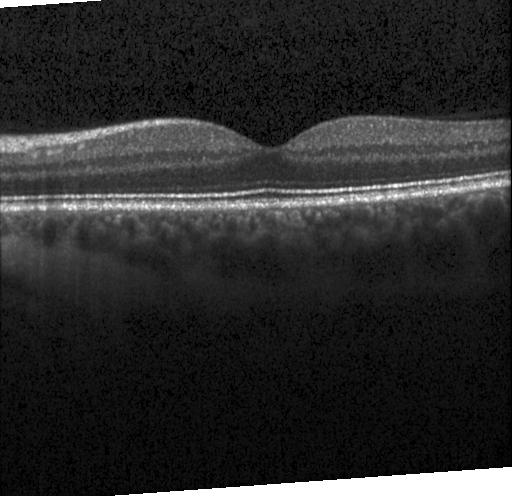
Retinal OCT B-scan.
Macular OCT: no choroidal neovascularization, diabetic macular edema, or drusen.